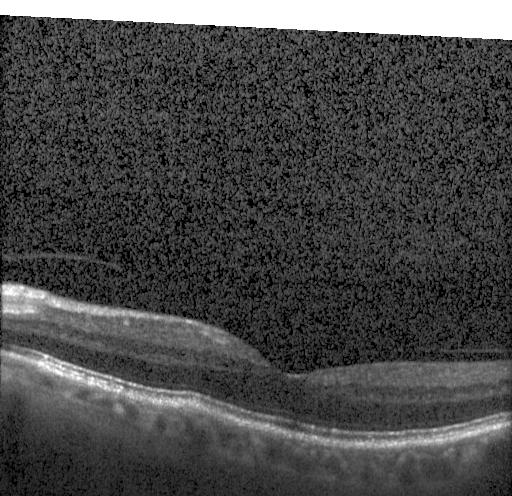
Fovea-centered, spectral-domain optical coherence tomography, OCT line scan
Dx: no choroidal neovascularization, no diabetic macular edema, and no drusen.